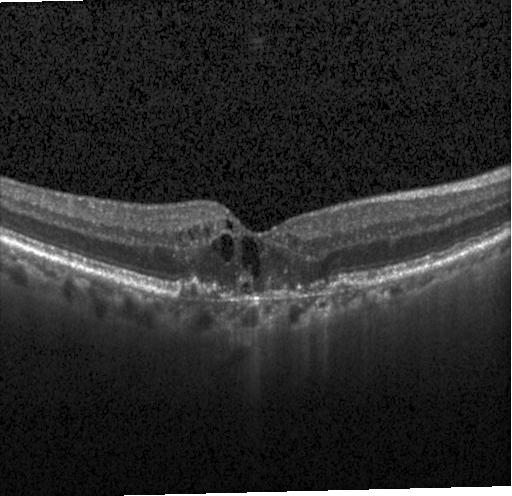

Diagnosis: choroidal neovascularization.